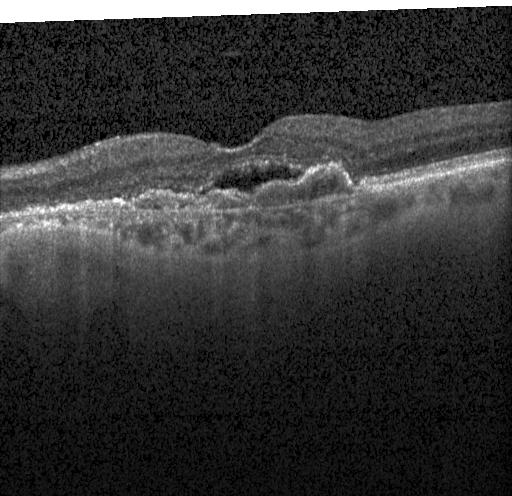
OCT line scan · Heidelberg Spectralis OCT system.
Diagnosis: CNV.